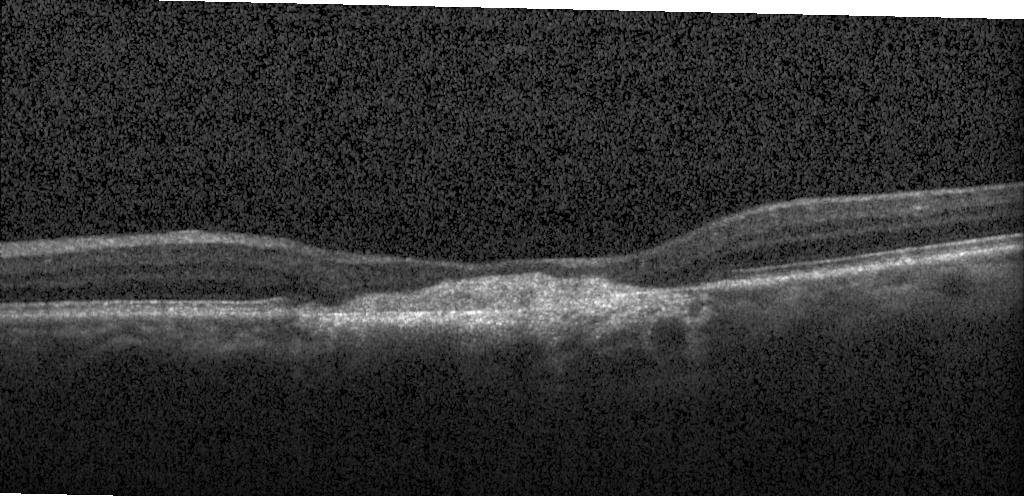

Diagnosis: a choroidal neovascular membrane.